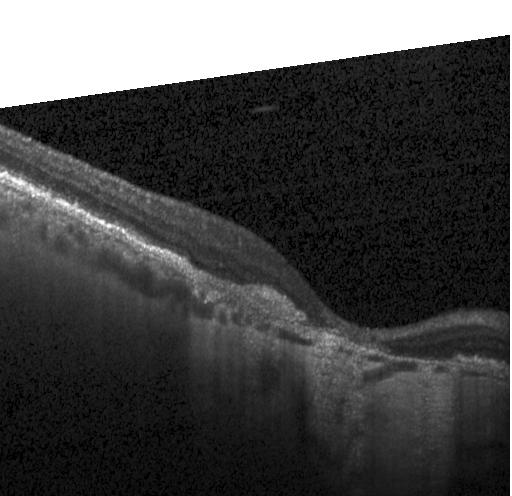 OCT line scan. SD-OCT.
Impression: CNV.